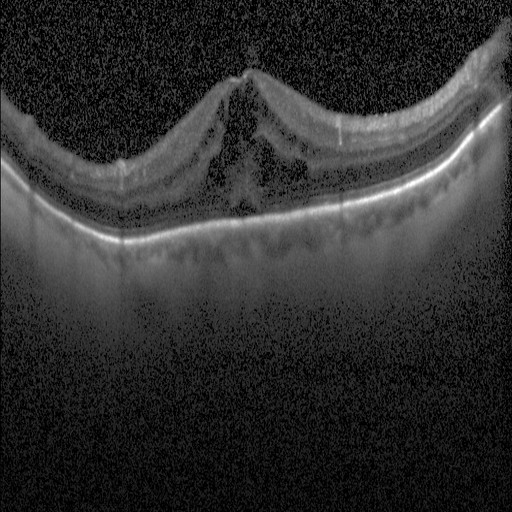
Diagnosis: diabetic macular edema (DME).